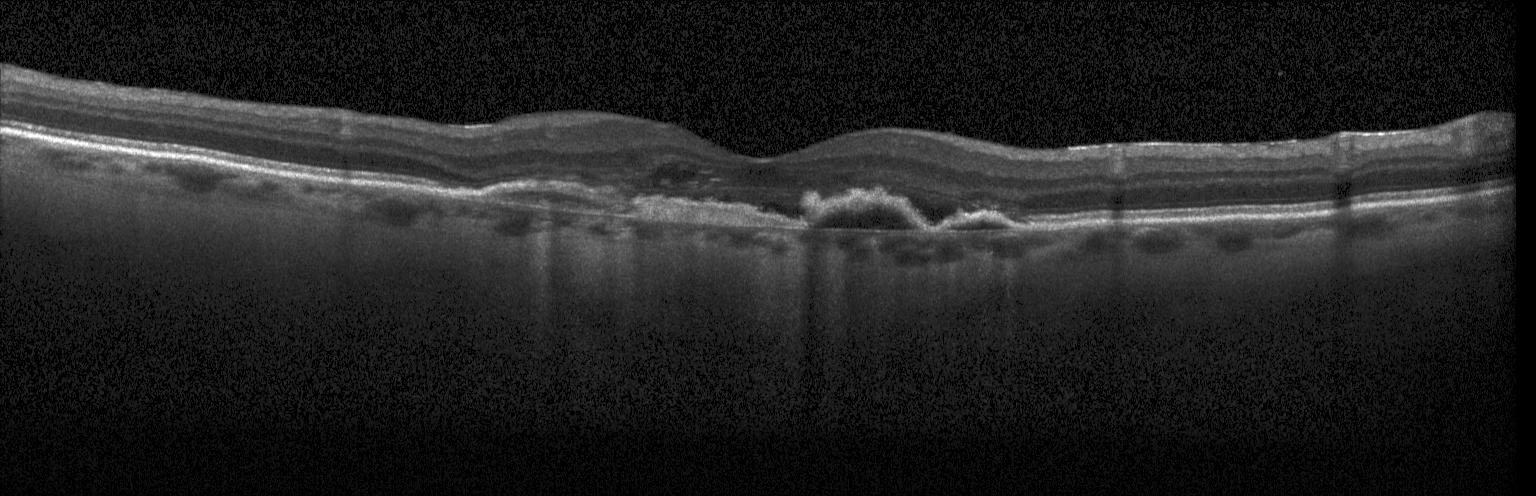

Dx: a choroidal neovascular membrane.